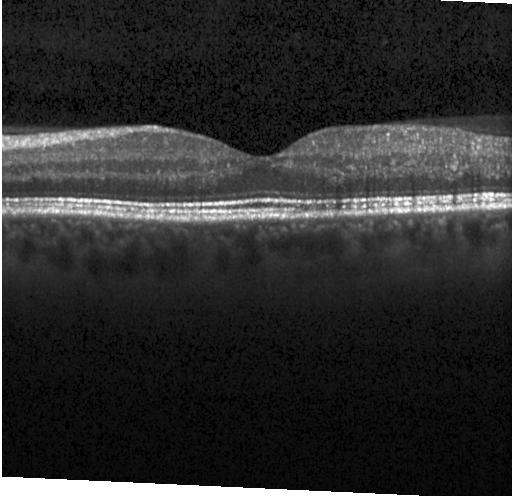
The scan shows no CNV, DME, or drusen.